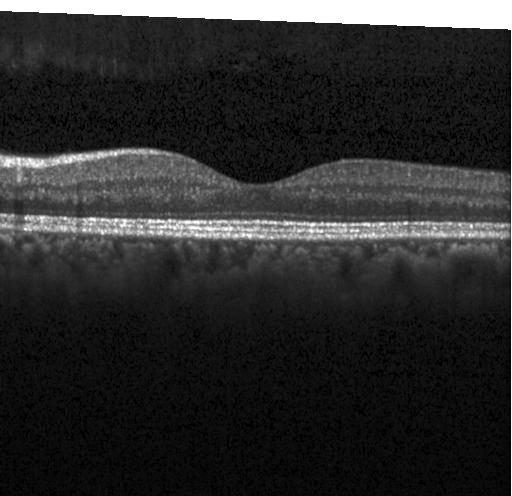
This B-scan demonstrates no evidence of CNV, DME, or drusen.